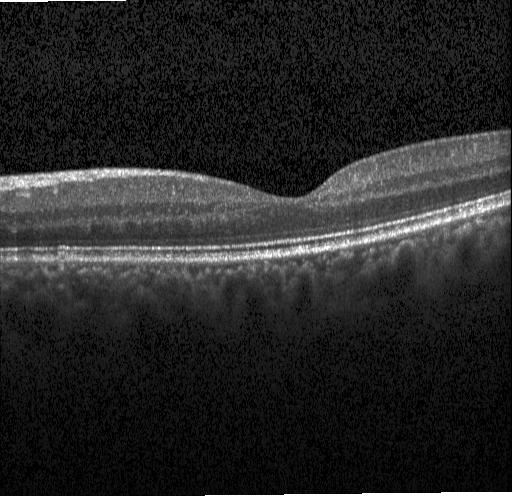

Heidelberg Spectralis, OCT B-scan. Impression: no CNV, no DME, and no drusen.